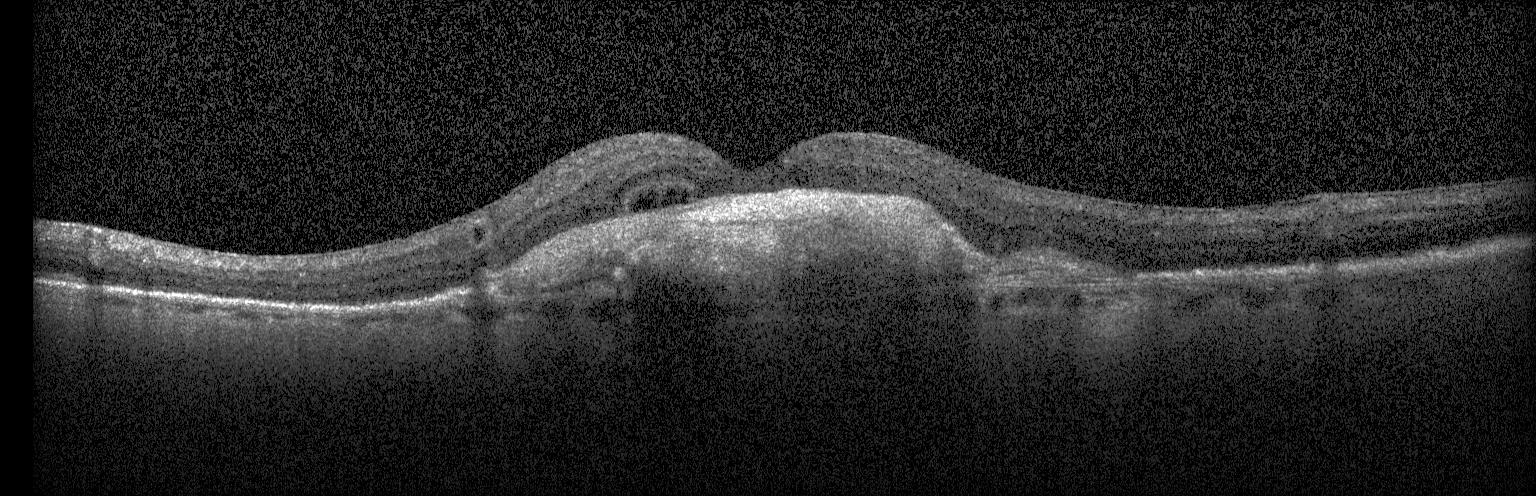
Macular OCT: a choroidal neovascular membrane.